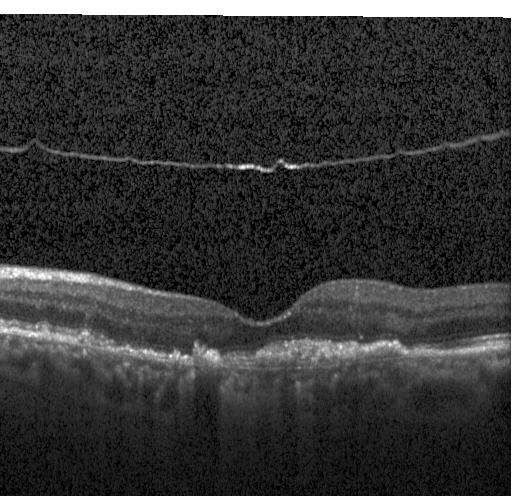

Heidelberg Spectralis, spectral-domain OCT, retinal OCT B-scan
Diagnosis: a choroidal neovascular membrane.